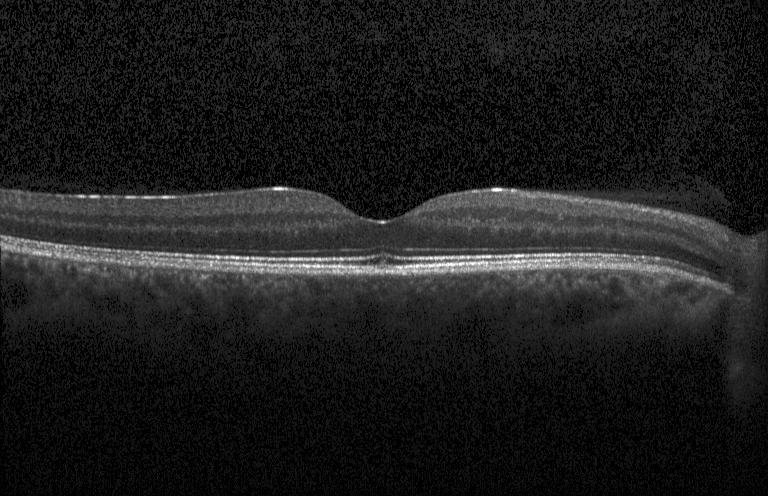

Acquired on a Heidelberg Spectralis. OCT B-scan
No evidence of CNV, DME, or drusen.